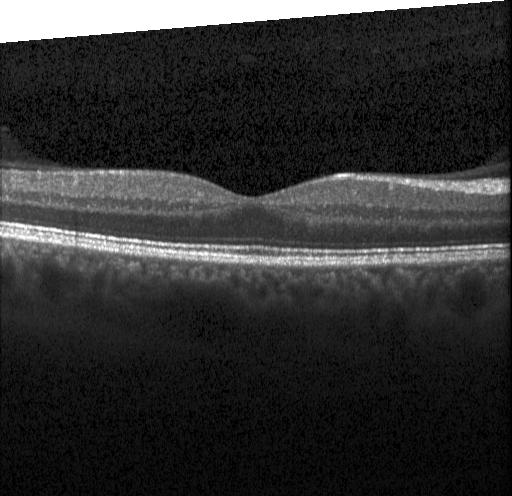 Instrument: Heidelberg Spectralis · optical coherence tomography scan — No choroidal neovascularization, diabetic macular edema, or drusen.